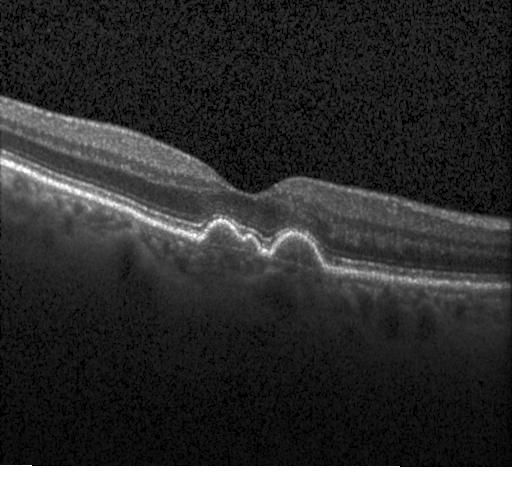 Macular scan; optical coherence tomography B-scan.
Impression: sub-RPE drusenoid deposits.